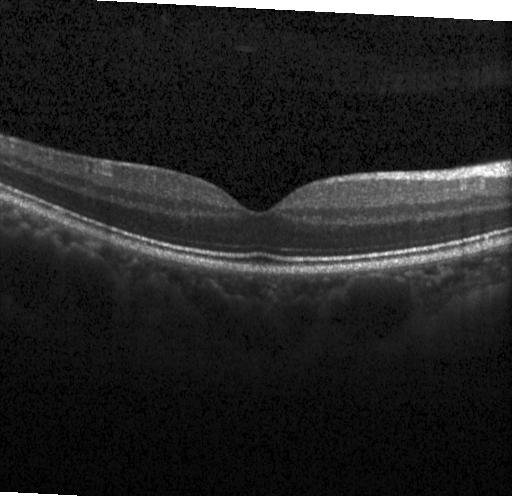

Optical coherence tomography scan. Through the macula — No CNV, DME, or drusen.